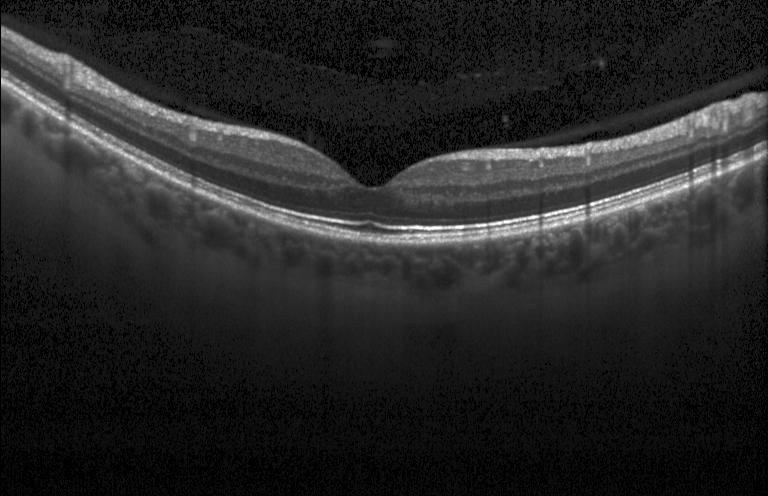

This B-scan demonstrates no choroidal neovascularization, diabetic macular edema, or drusen.